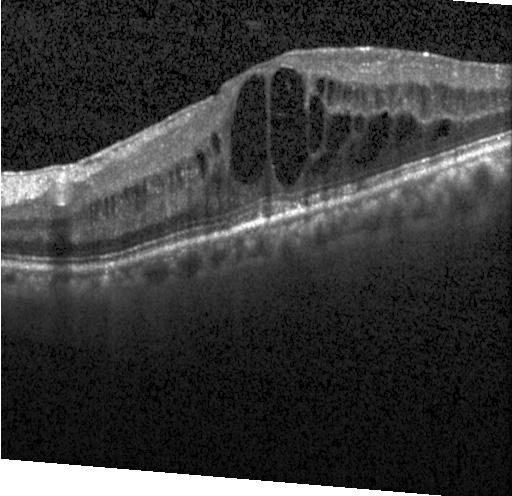

Optical coherence tomography B-scan. Centered on the fovea. Impression: DME.